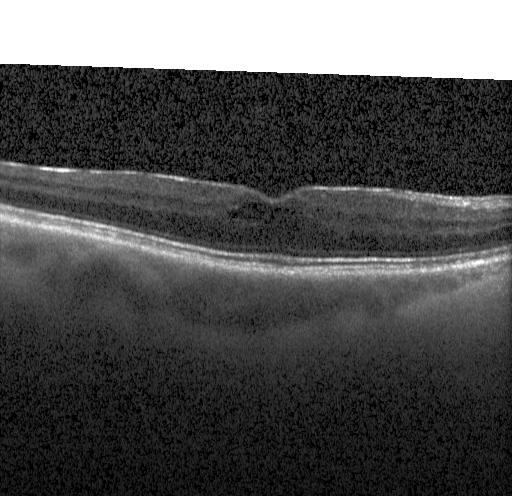

Optical coherence tomography scan; SD-OCT; through the macula; Heidelberg Spectralis — Dx: diabetic macular edema.